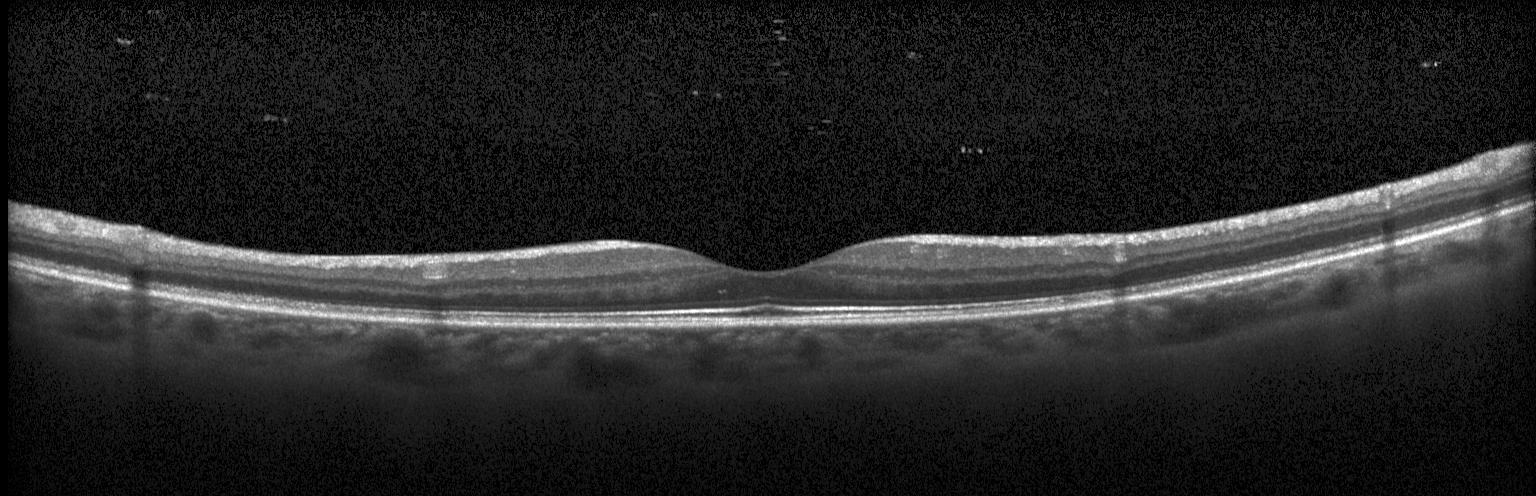

OCT B-scan
Diagnosis: neither choroidal neovascularization, diabetic macular edema, nor drusen.